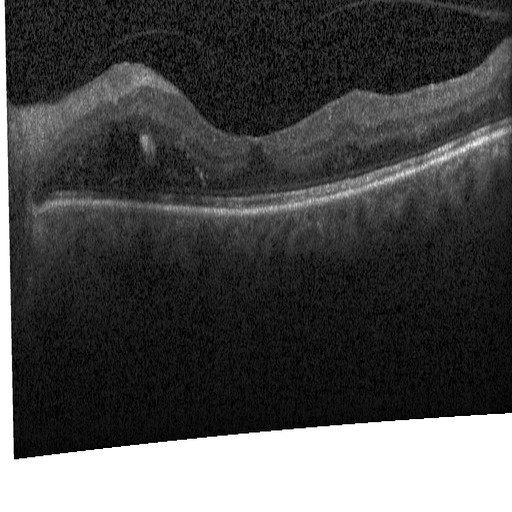

Macular scan, OCT line scan
OCT finding: diabetic macular edema (DME).